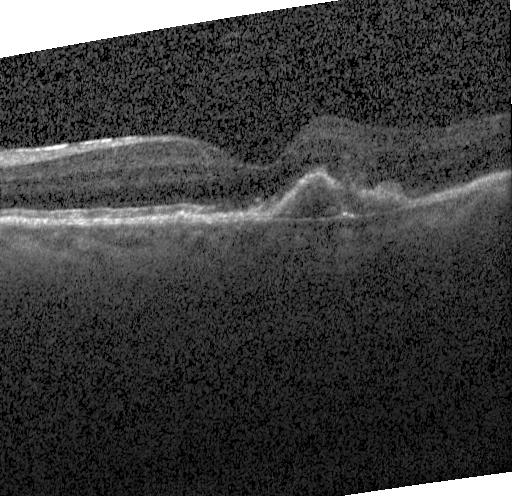
OCT line scan — The scan shows a choroidal neovascular membrane.